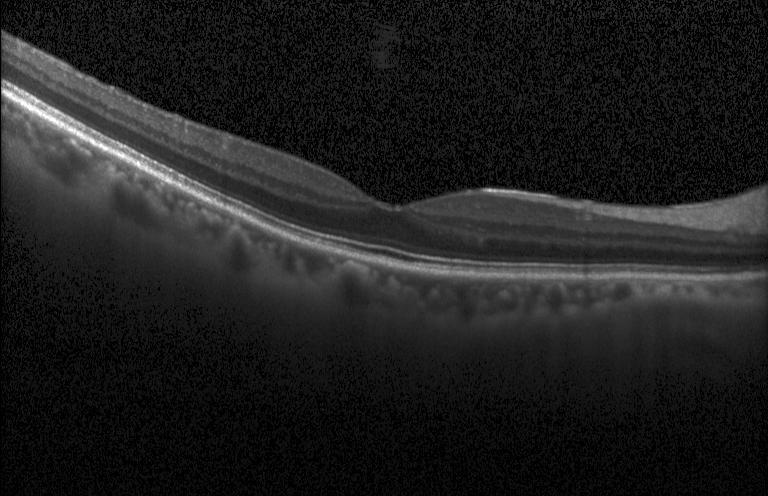
Spectral-domain OCT B-scan: neither CNV, DME, nor drusen.